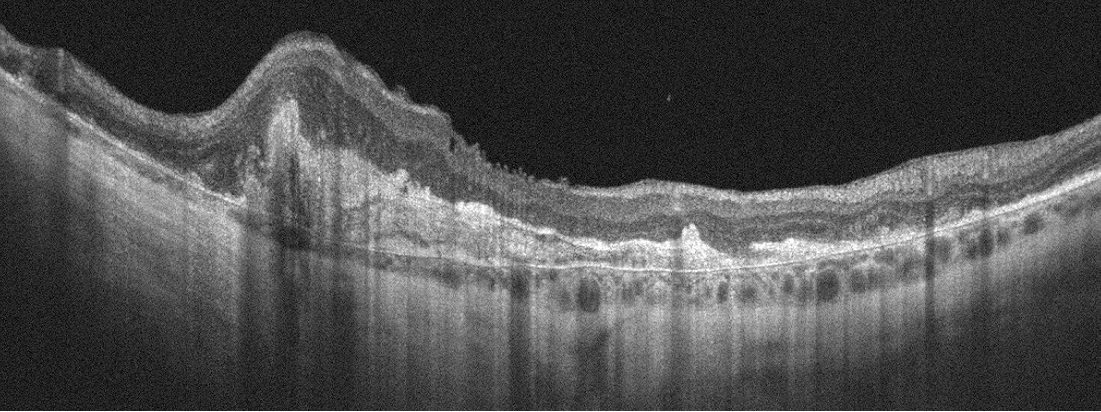
Acquired on an Optovue Avanti RTVue XR; retinal OCT cross-section.
Diagnosis: AMD.